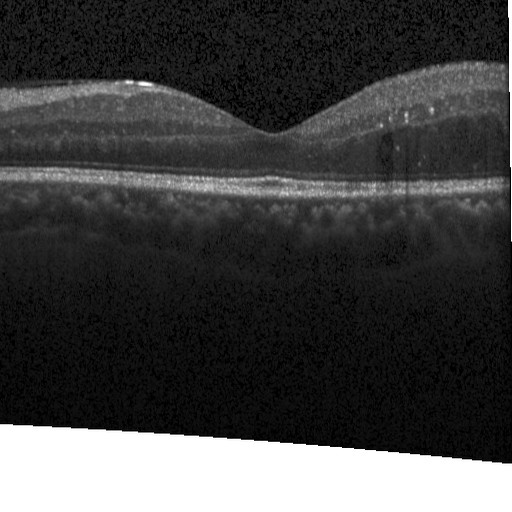

Retinal OCT cross-section. Finding: diabetic macular edema (DME).